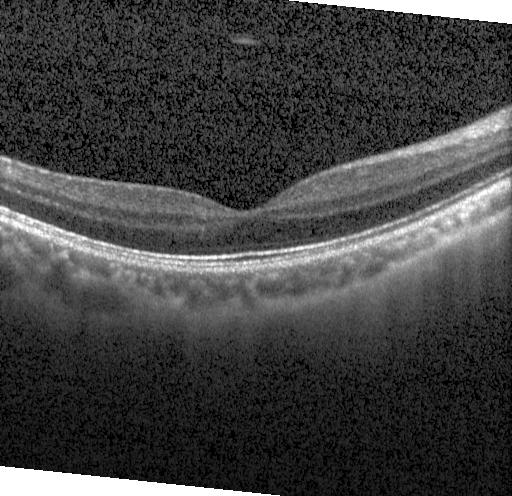
Optical coherence tomography scan — Finding: neither choroidal neovascularization, diabetic macular edema, nor drusen.